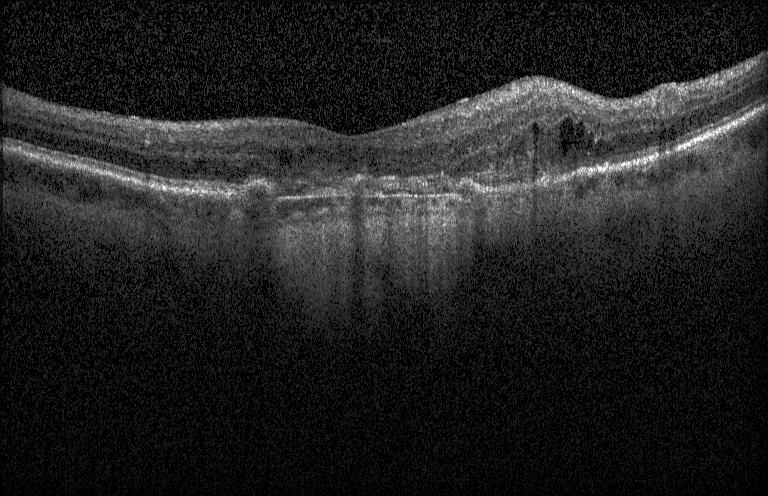
Retinal OCT cross-section, Heidelberg Spectralis OCT system
Impression: CNV.